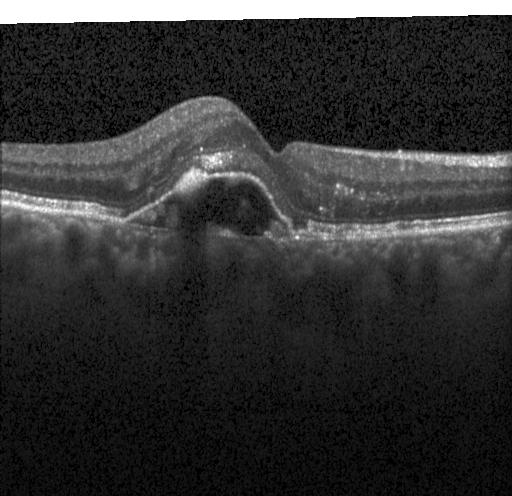
SD-OCT, OCT B-scan, macular scan — Finding: a choroidal neovascular membrane.